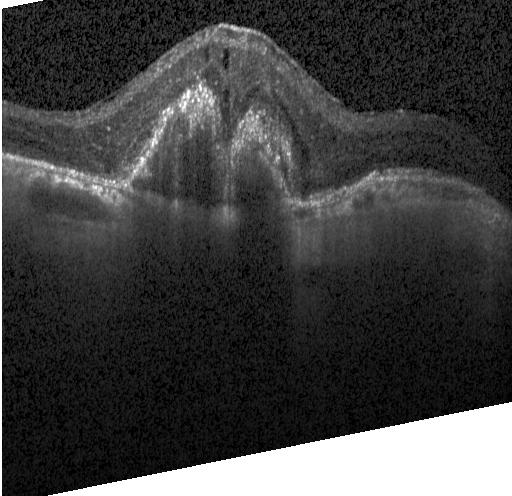

Heidelberg Spectralis; optical coherence tomography B-scan.
Impression: choroidal neovascularization (CNV).